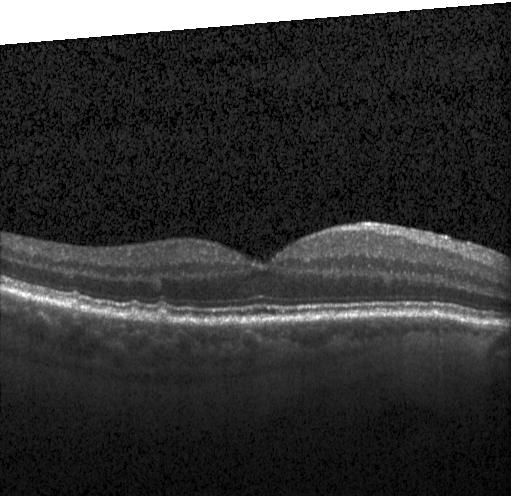
Through the macula; spectral-domain OCT; OCT line scan; acquired on a Heidelberg Spectralis.
This B-scan demonstrates sub-RPE drusenoid deposits.